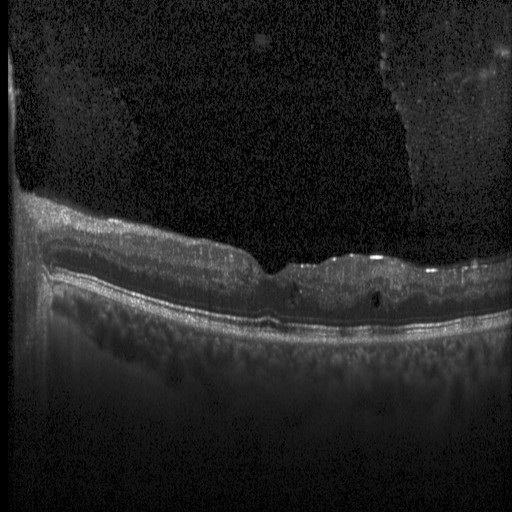
Diagnosis: diabetic macular edema (DME).